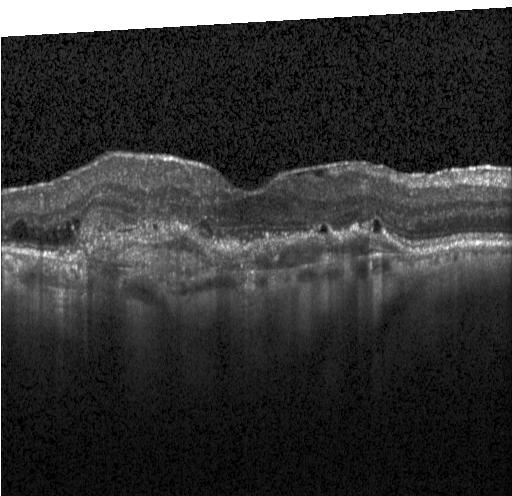

Fovea-centered · spectral-domain optical coherence tomography · optical coherence tomography scan — Impression: CNV.